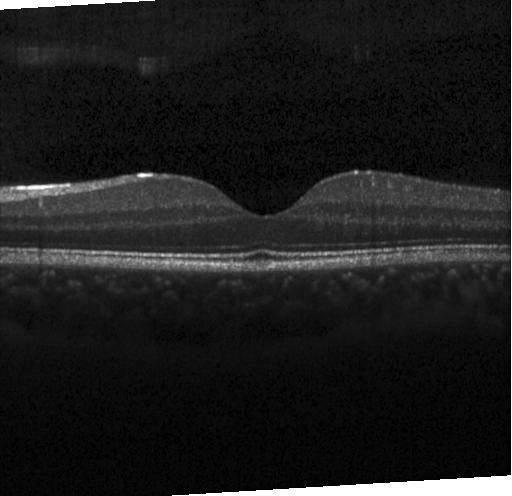
Retinal OCT cross-section. Fovea-centered. Spectral-domain optical coherence tomography — No choroidal neovascularization, no diabetic macular edema, and no drusen.